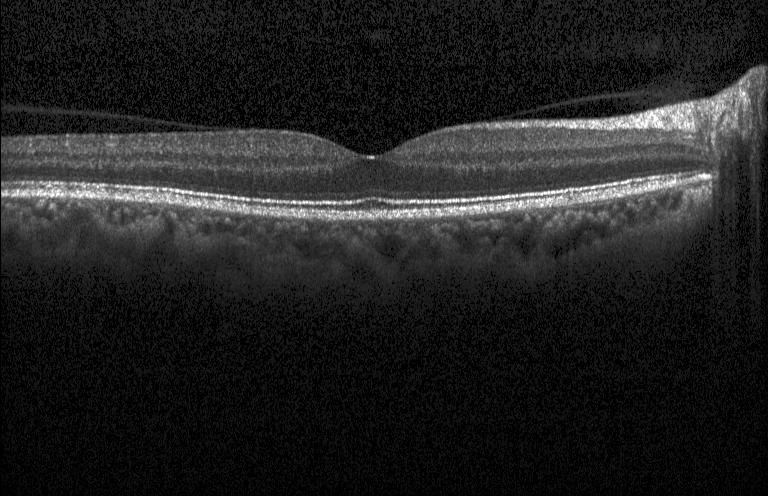

OCT B-scan showing no CNV, no DME, and no drusen.